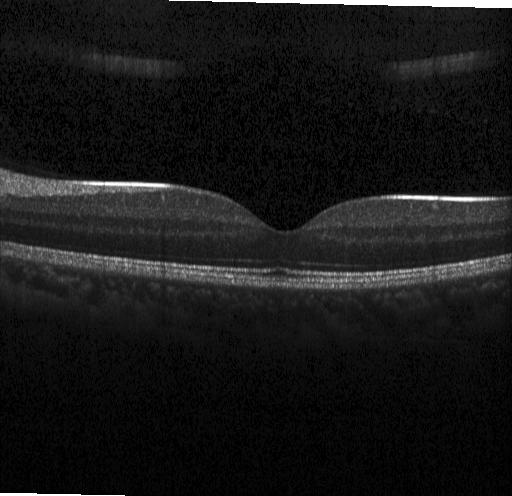 The scan shows no evidence of CNV, DME, or drusen.